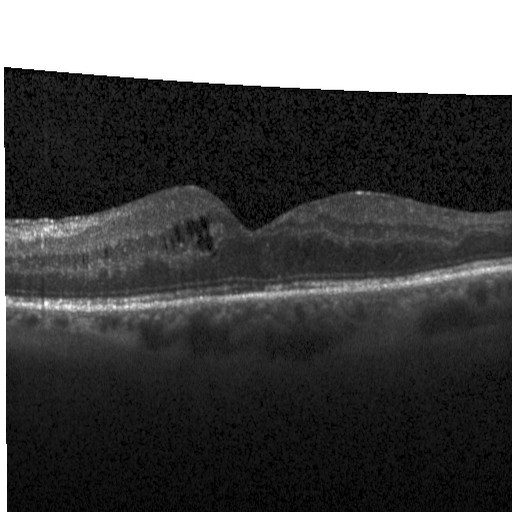
OCT B-scan.
Impression: diabetic macular edema.